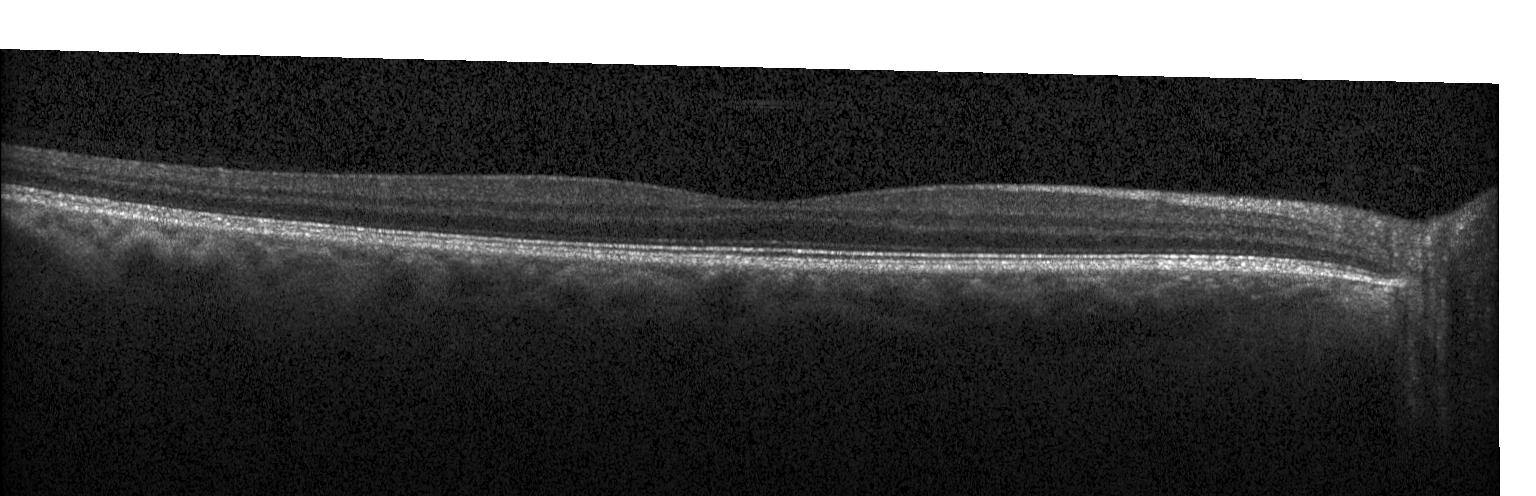
Impression: no choroidal neovascularization, no diabetic macular edema, and no drusen.